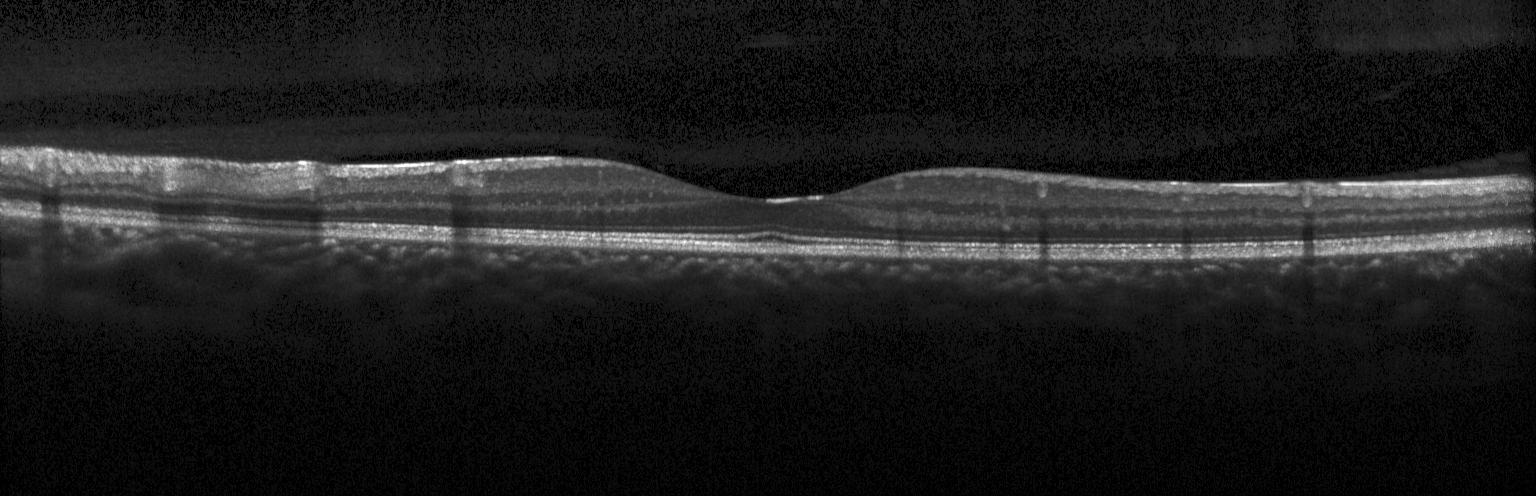 Macular OCT demonstrating no evidence of choroidal neovascularization, diabetic macular edema, or drusen.